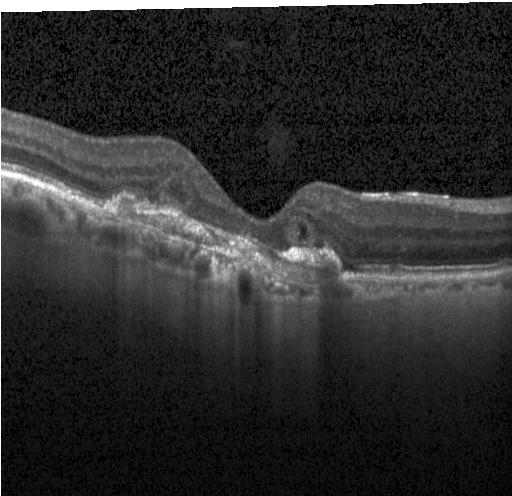

Retinal OCT B-scan · horizontal scan through the fovea · Heidelberg Spectralis
The scan shows a choroidal neovascular membrane.